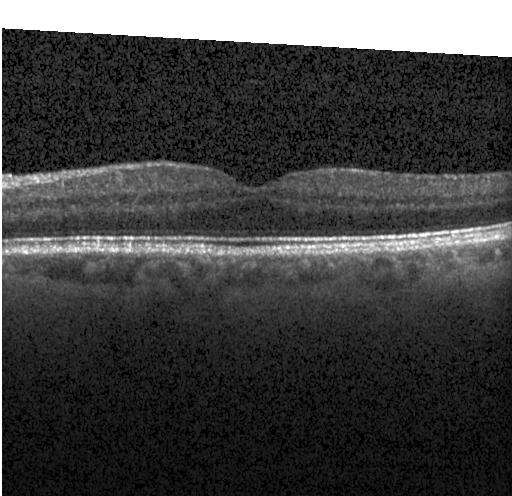 OCT line scan. Spectral-domain optical coherence tomography. Through the macula. Instrument: Heidelberg Spectralis
OCT finding: no CNV, DME, or drusen.